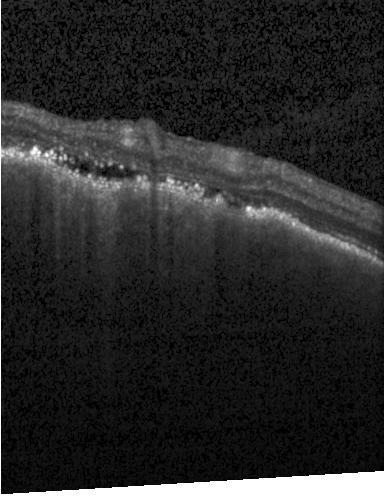

Retinal OCT cross-section
Finding: a choroidal neovascular membrane.